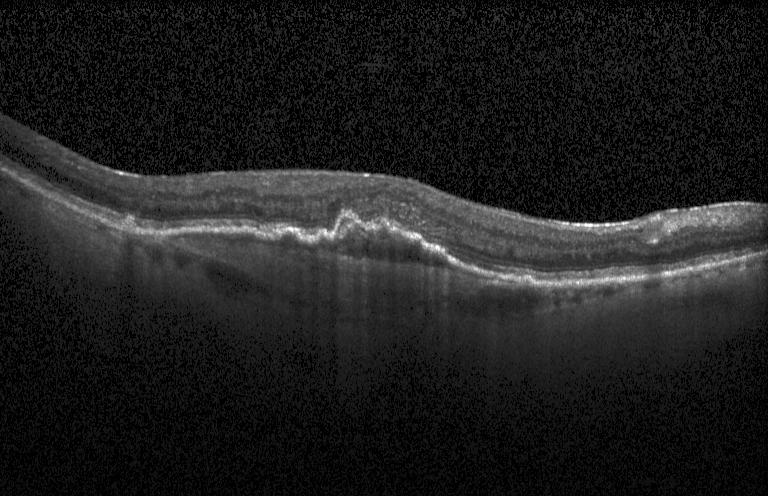

Finding: a choroidal neovascular membrane.